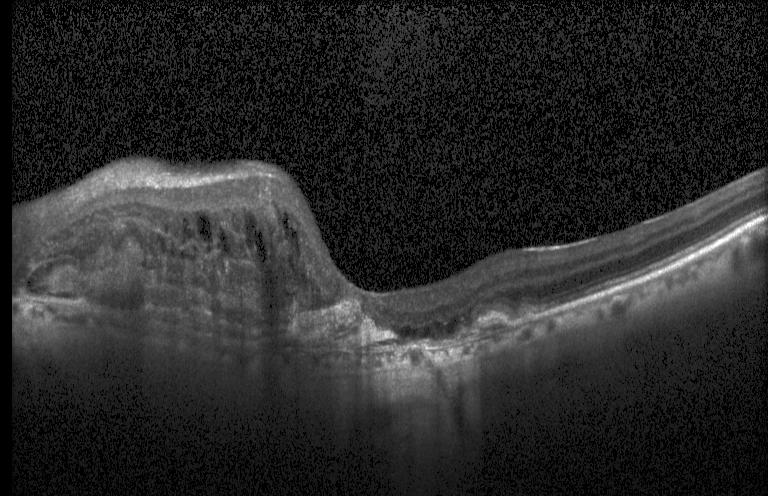
Impression: choroidal neovascularization (CNV).